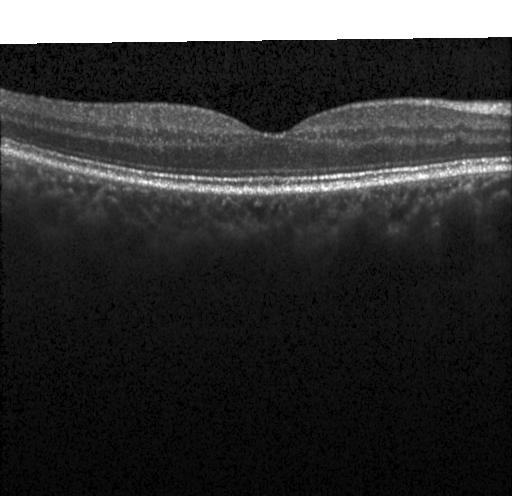 Impression: neither CNV, DME, nor drusen.